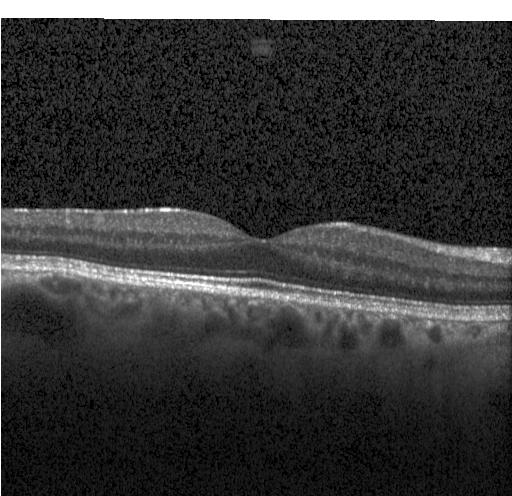 Retinal OCT cross-section.
Dx: neither choroidal neovascularization, diabetic macular edema, nor drusen.